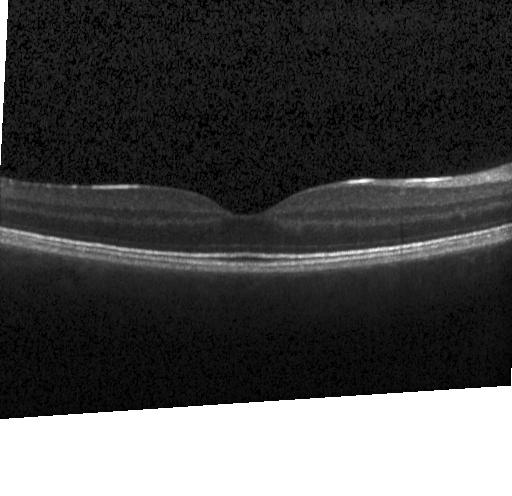 Spectral-domain OCT, horizontal scan through the fovea, optical coherence tomography scan. Finding: no choroidal neovascularization, no diabetic macular edema, and no drusen.